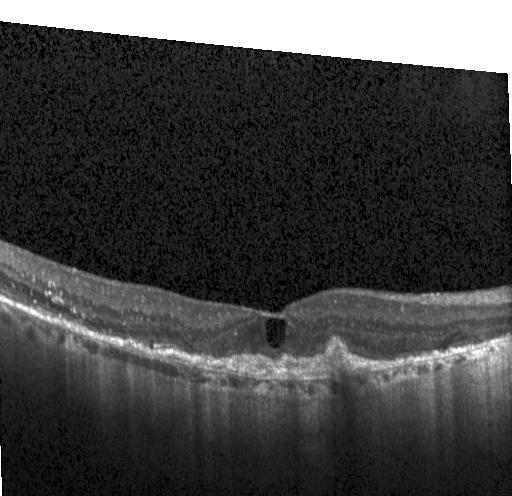

OCT B-scan, centered on the fovea — Impression: choroidal neovascularization.